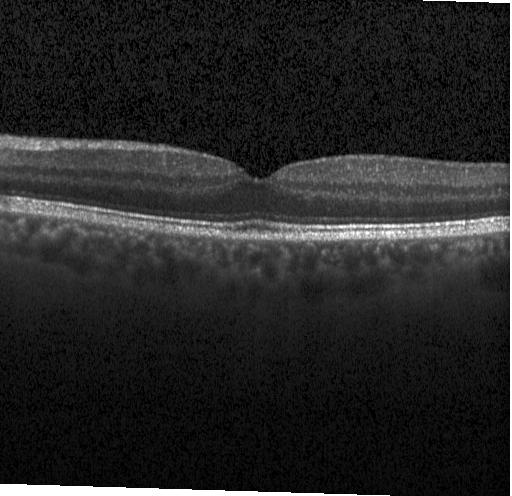 Centered on the fovea; optical coherence tomography scan.
Diagnosis: no choroidal neovascularization, diabetic macular edema, or drusen.